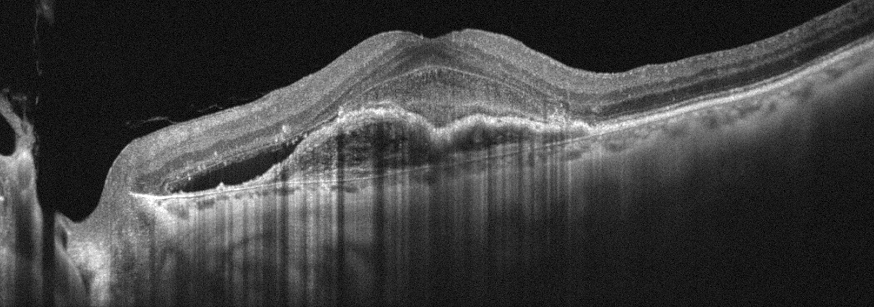
Optovue Avanti RTVue XR. Retinal OCT B-scan.
Assessment: age-related macular degeneration.